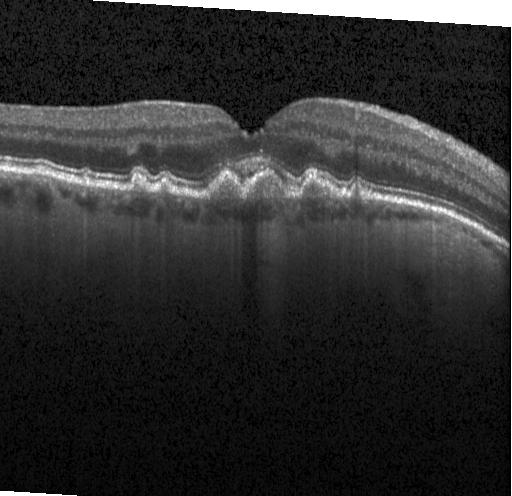 SD-OCT, retinal OCT cross-section
This B-scan demonstrates multiple drusen.